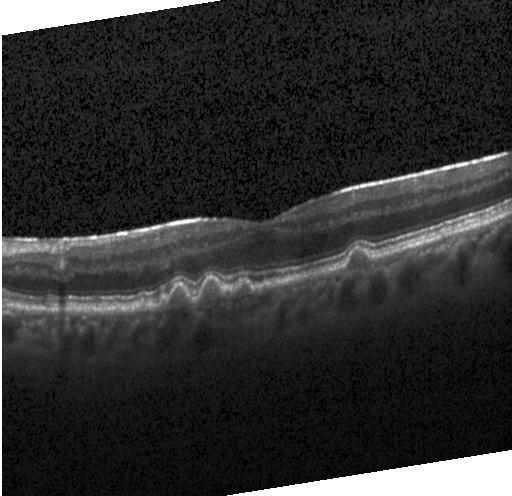
OCT B-scan.
Impression: drusen.